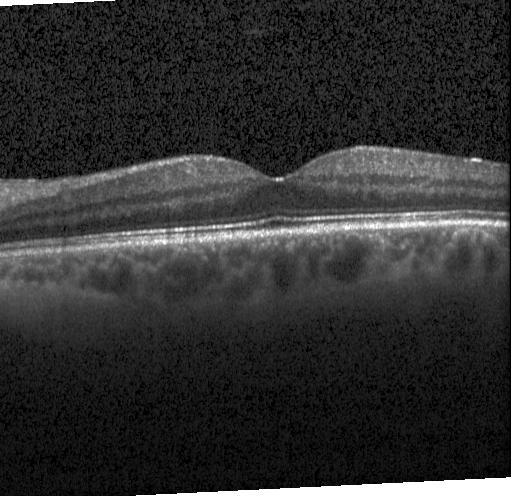

Instrument: Heidelberg Spectralis · retinal OCT B-scan · SD-OCT — Diagnosis: no CNV, no DME, and no drusen.